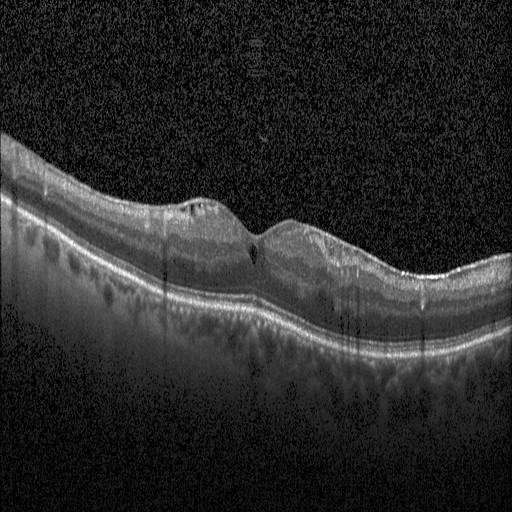
Macular scan; spectral-domain optical coherence tomography; retinal OCT B-scan.
Diagnosis: diabetic macular edema.